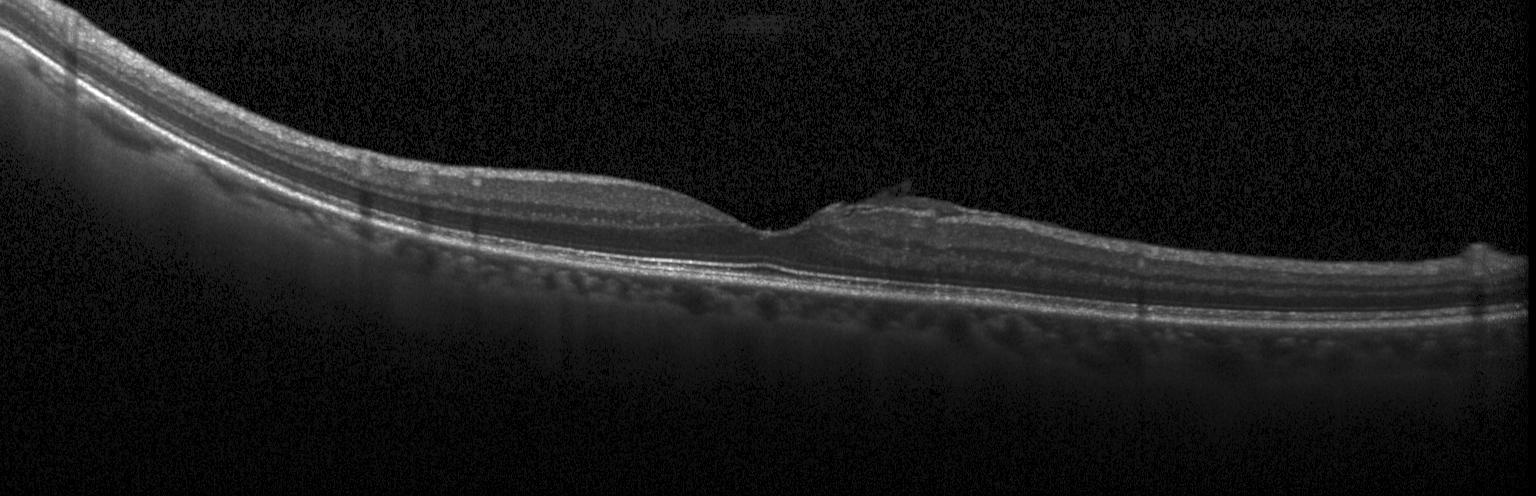

Diagnosis: no CNV, no DME, and no drusen.